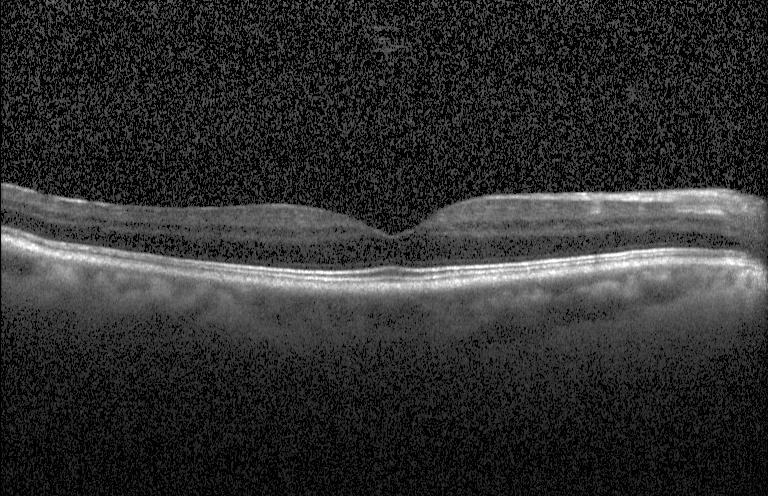
Impression: neither choroidal neovascularization, diabetic macular edema, nor drusen.